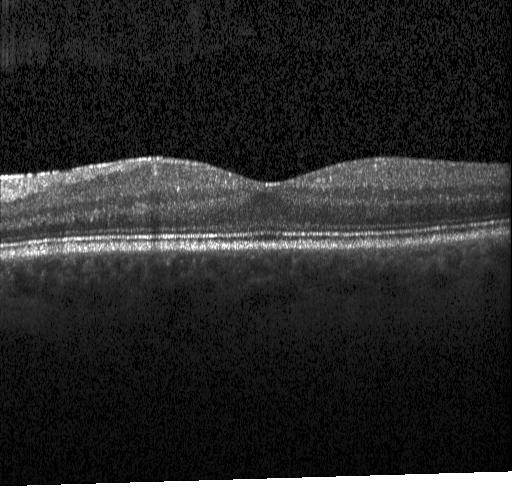

OCT scan showing no evidence of choroidal neovascularization, diabetic macular edema, or drusen.